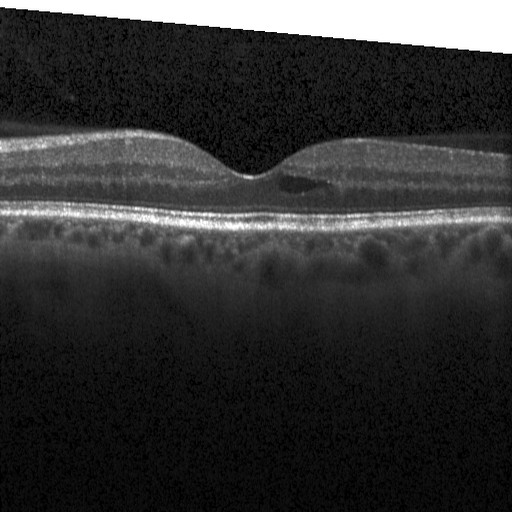 Acquired on a Heidelberg Spectralis · OCT B-scan — Finding: diabetic macular edema (DME).